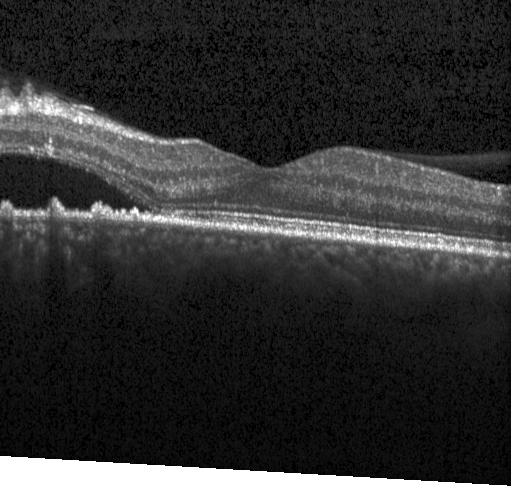

OCT B-scan. Diagnosis: a choroidal neovascular membrane.